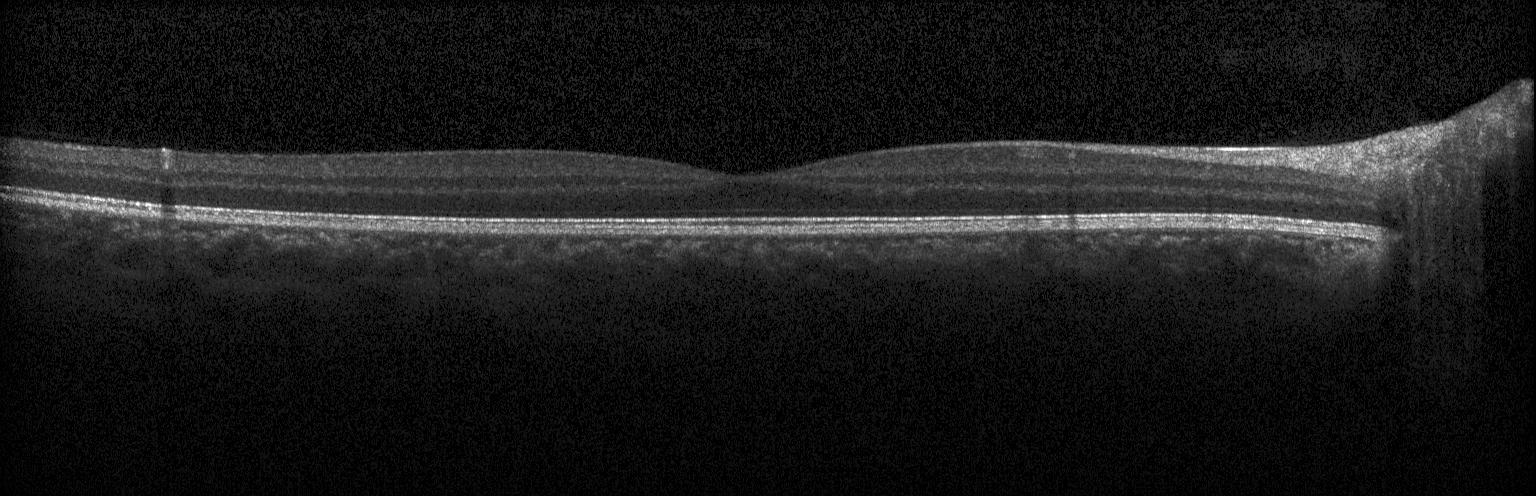
Impression: no CNV, no DME, and no drusen.